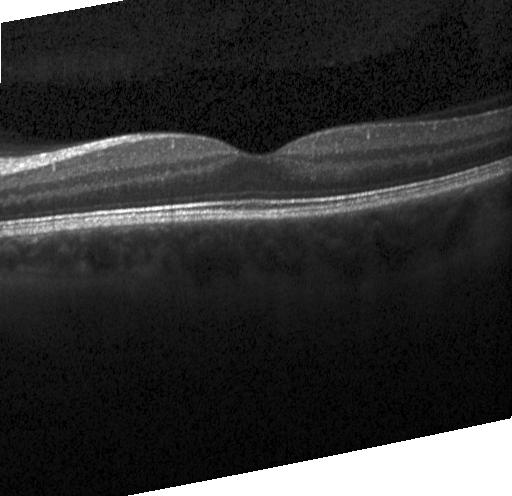
Finding: no CNV, DME, or drusen.